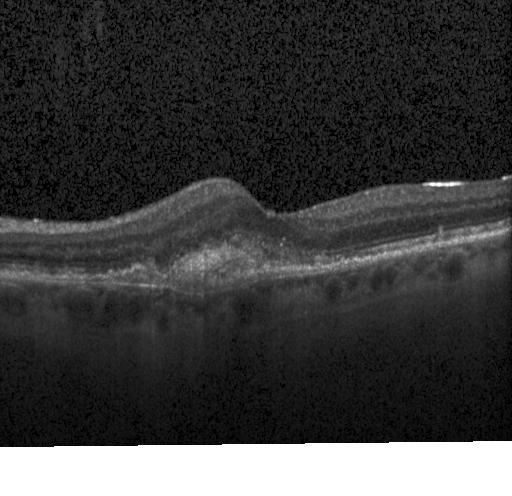 Finding: a choroidal neovascular membrane.